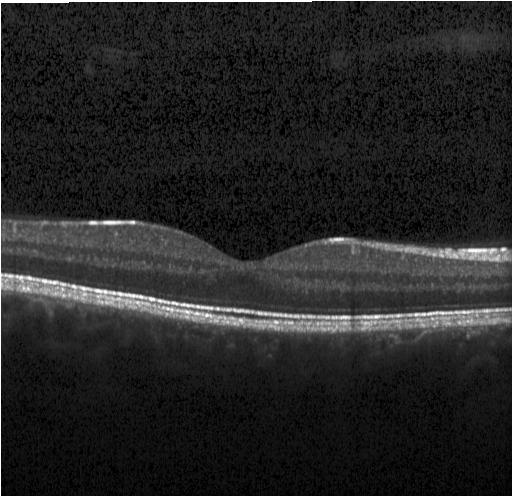 OCT B-scan.
Impression: no CNV, no DME, and no drusen.